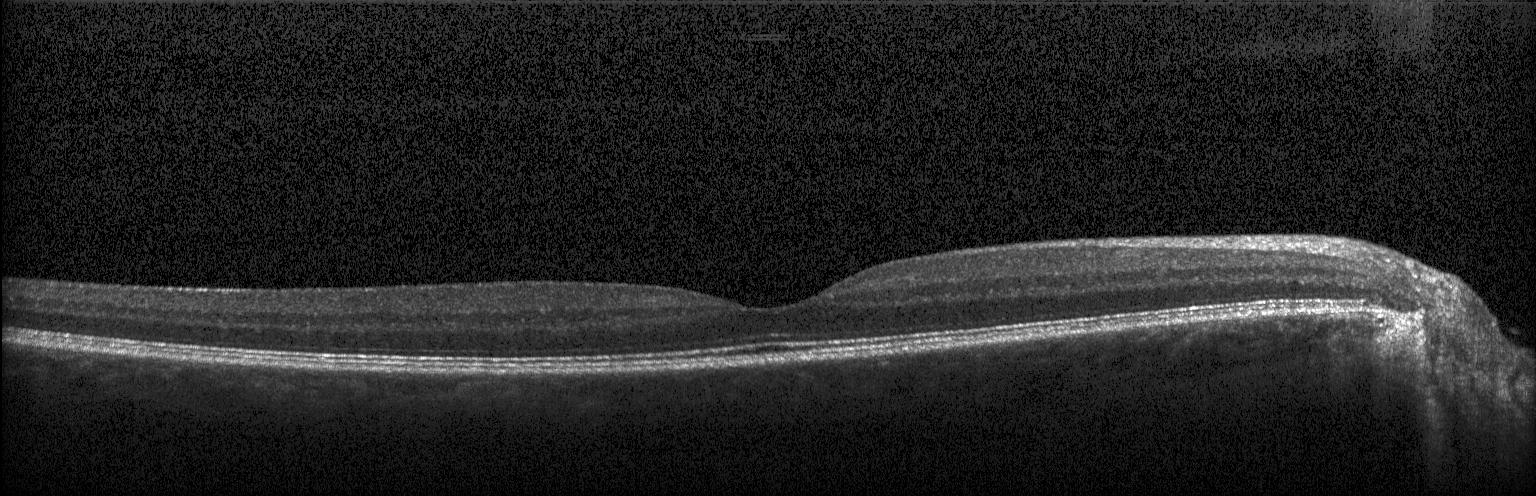 Retinal OCT cross-section showing neither CNV, DME, nor drusen.